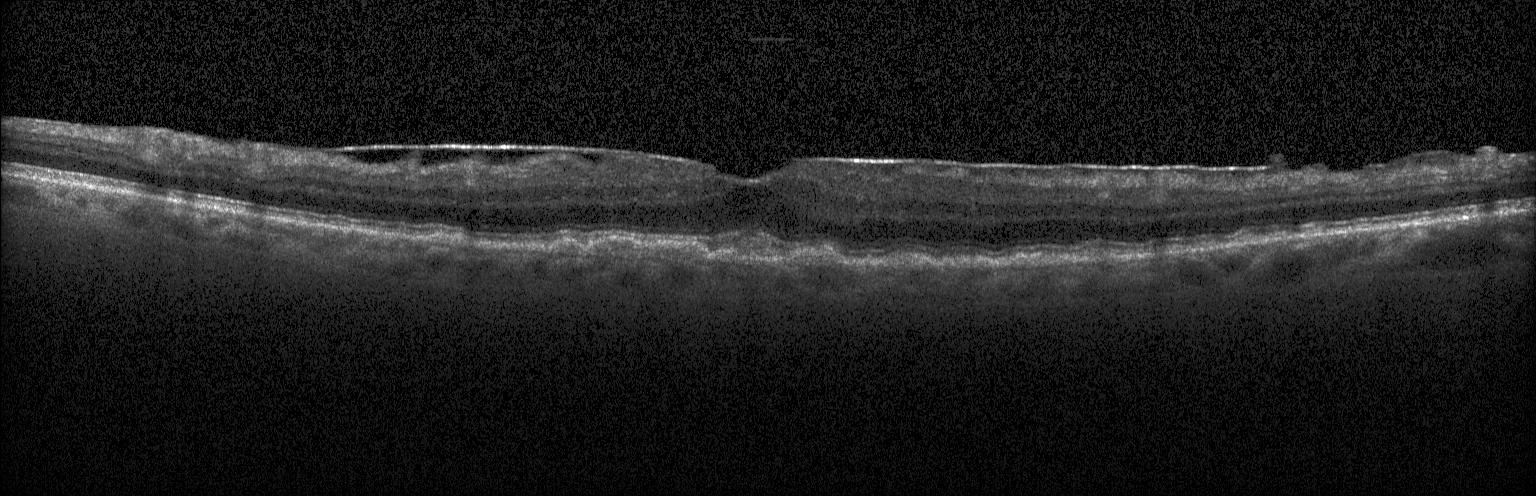

This B-scan demonstrates multiple drusen.